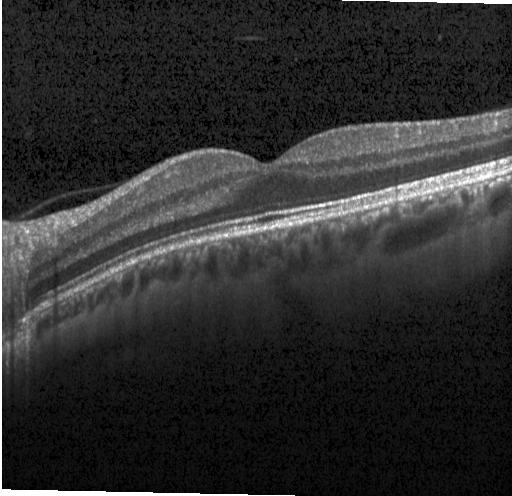
Diagnosis: no evidence of CNV, DME, or drusen.